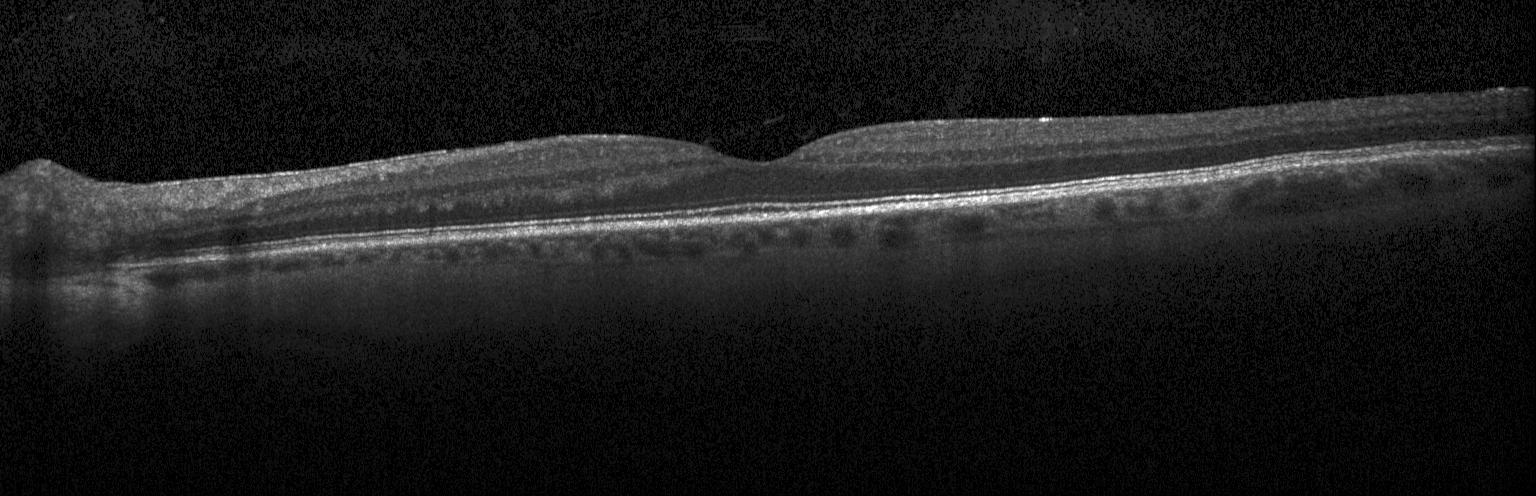
This B-scan demonstrates no choroidal neovascularization, diabetic macular edema, or drusen.